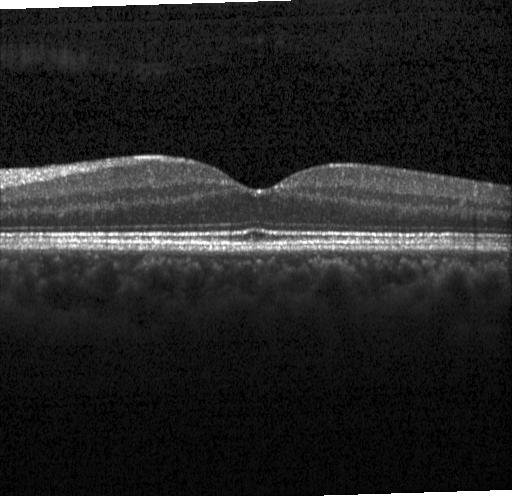
Assessment: no CNV, no DME, and no drusen.